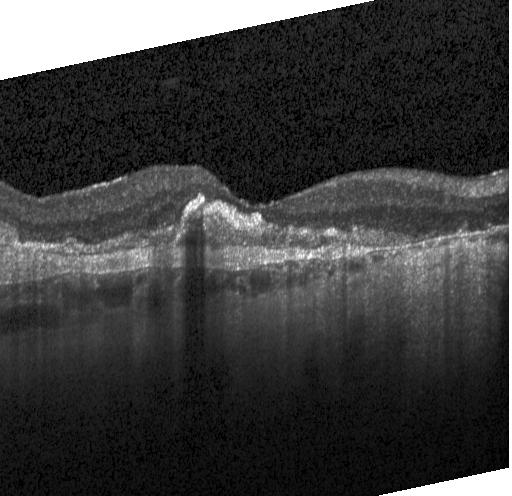

Optical coherence tomography B-scan — Diagnosis: a choroidal neovascular membrane.